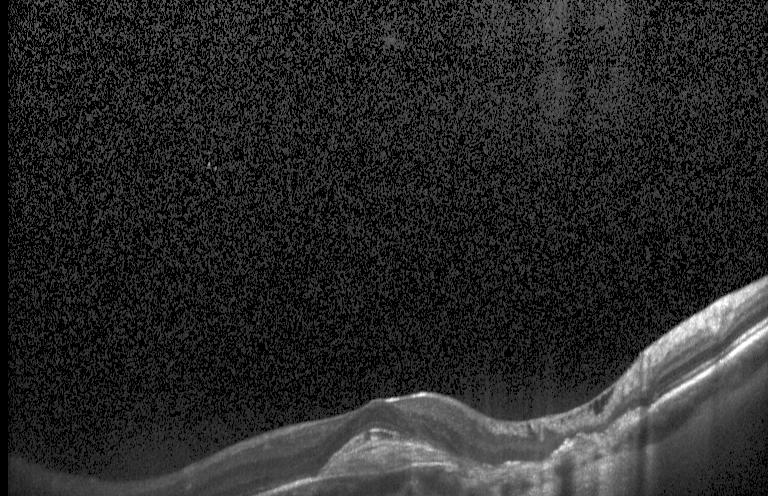 Spectral-domain OCT; centered on the fovea; optical coherence tomography scan.
CNV.